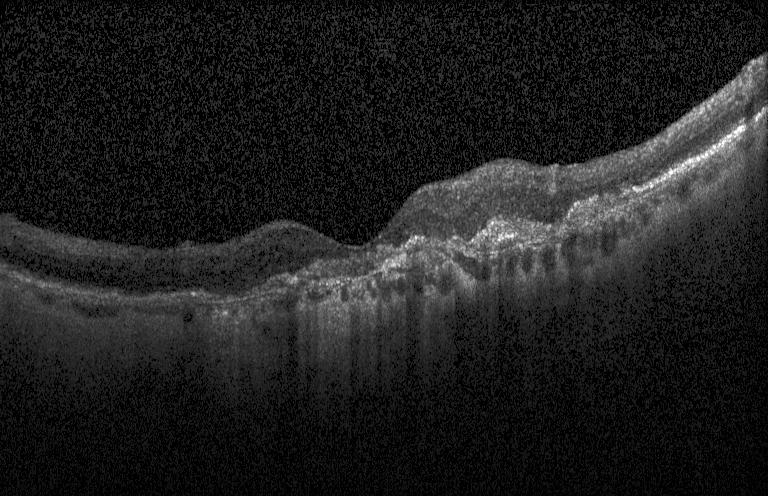 OCT line scan, fovea-centered
The scan shows a choroidal neovascular membrane.